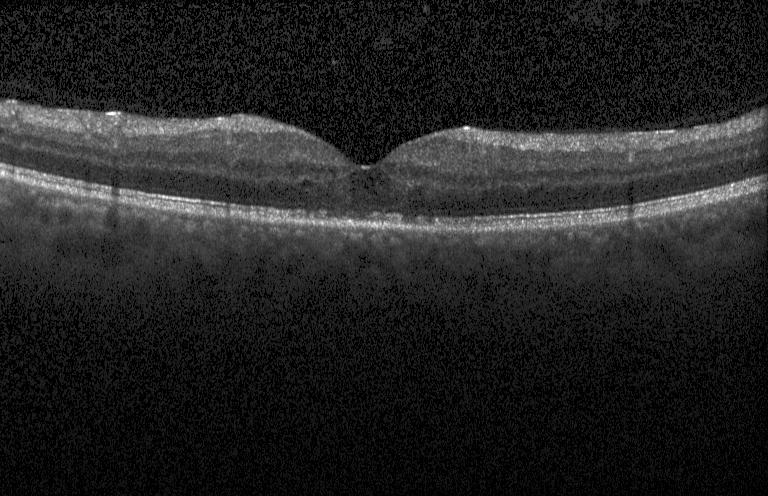
OCT line scan; horizontal scan through the fovea.
The scan shows DME.